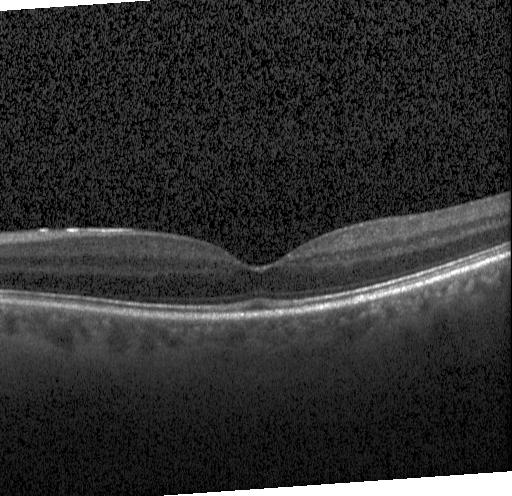

Impression: neither CNV, DME, nor drusen.